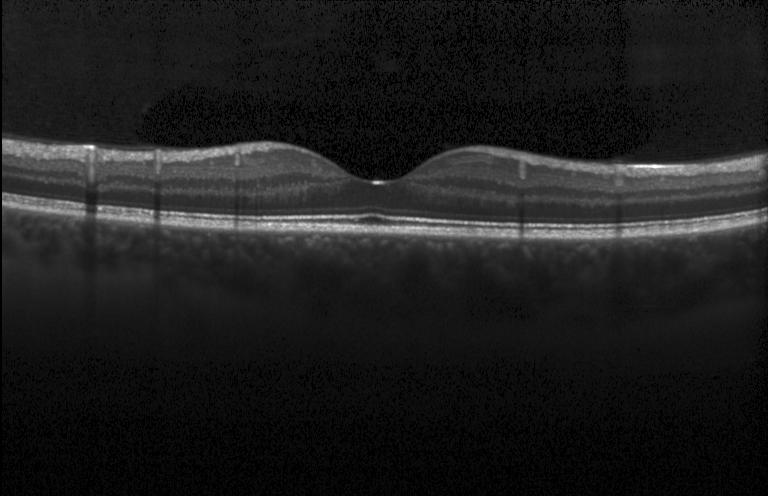
Assessment: no choroidal neovascularization, no diabetic macular edema, and no drusen.